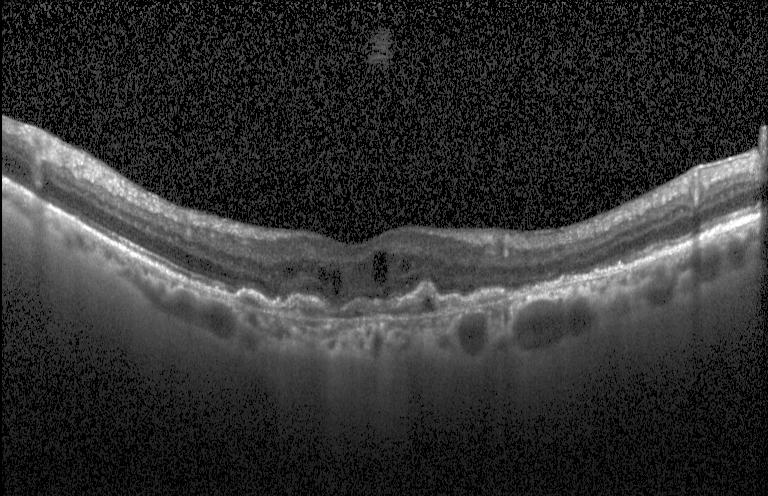

OCT B-scan
OCT finding: a choroidal neovascular membrane.